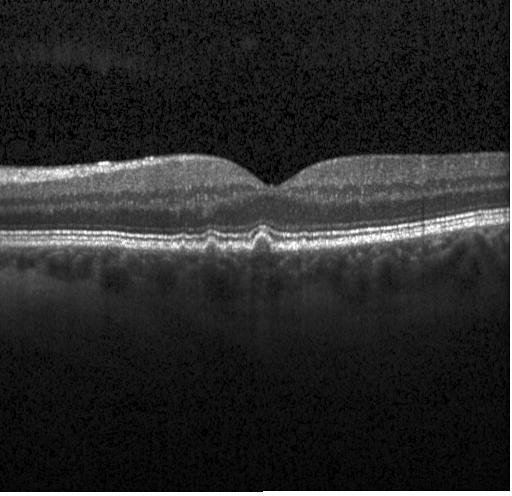
Horizontal scan through the fovea; OCT line scan; spectral-domain OCT; Heidelberg Spectralis OCT system. Drusen.